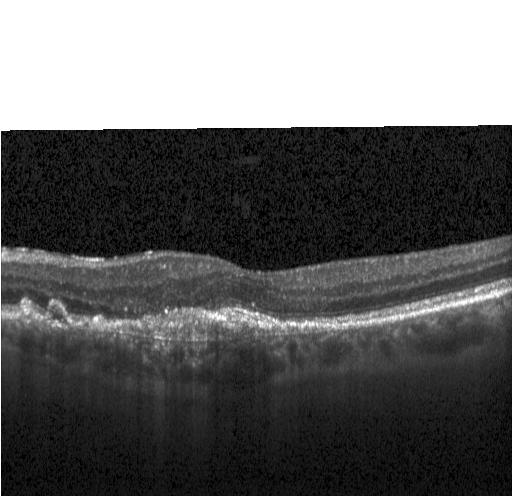
Horizontal scan through the fovea. Heidelberg Spectralis. Optical coherence tomography scan.
Finding: choroidal neovascularization.